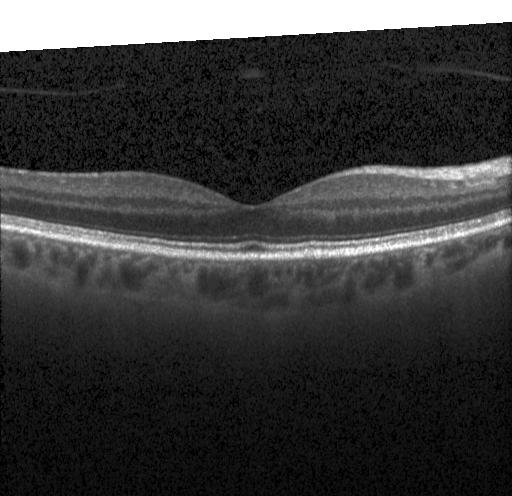
OCT line scan, through the macula. Impression: no choroidal neovascularization, diabetic macular edema, or drusen.